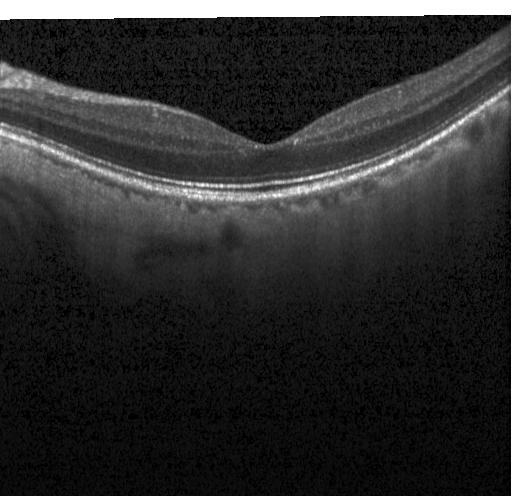

Impression: no choroidal neovascularization, no diabetic macular edema, and no drusen.